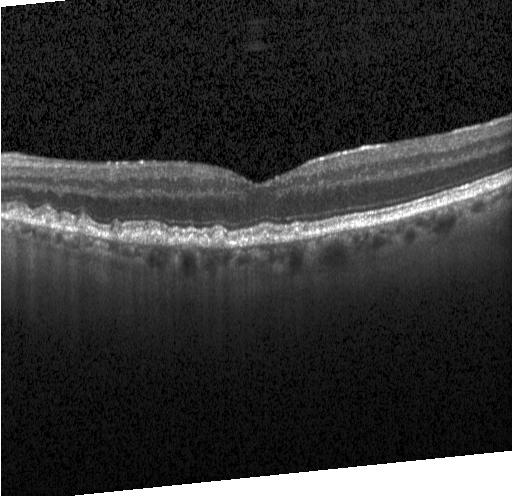
OCT finding: drusen.